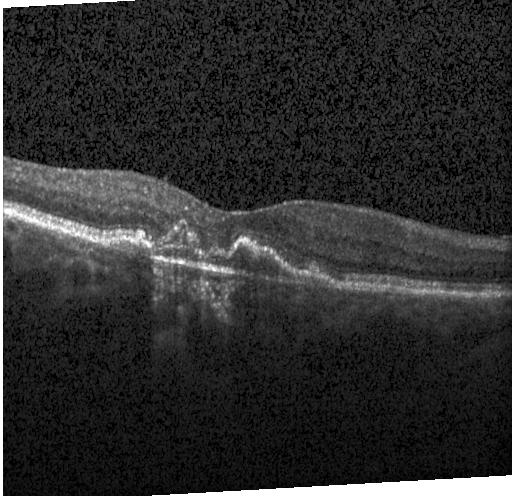

OCT scan showing choroidal neovascularization.